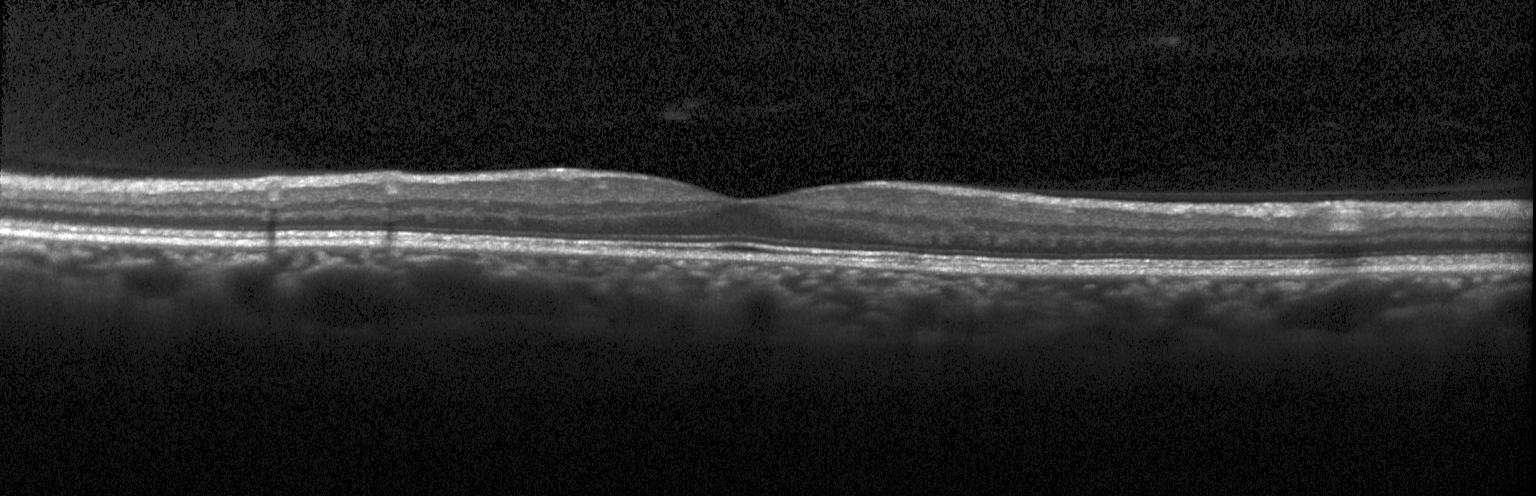

OCT finding: no choroidal neovascularization, no diabetic macular edema, and no drusen.